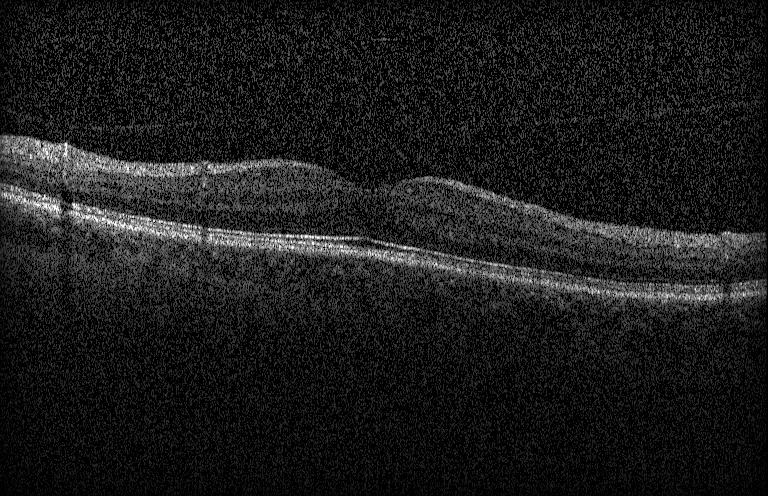 Retinal OCT cross-section · spectral-domain OCT. The scan shows no choroidal neovascularization, diabetic macular edema, or drusen.